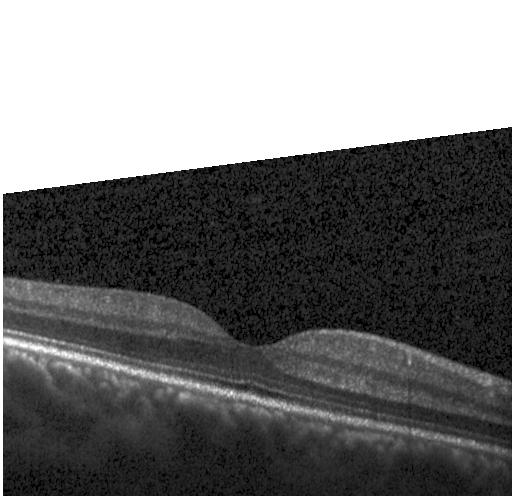

Through the macula, retinal OCT cross-section, Heidelberg Spectralis.
This B-scan demonstrates no choroidal neovascularization, diabetic macular edema, or drusen.